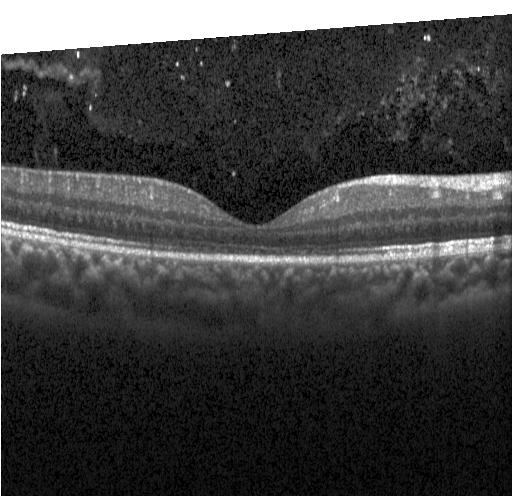

Instrument: Heidelberg Spectralis. Optical coherence tomography scan. SD-OCT. Through the macula — Impression: neither choroidal neovascularization, diabetic macular edema, nor drusen.